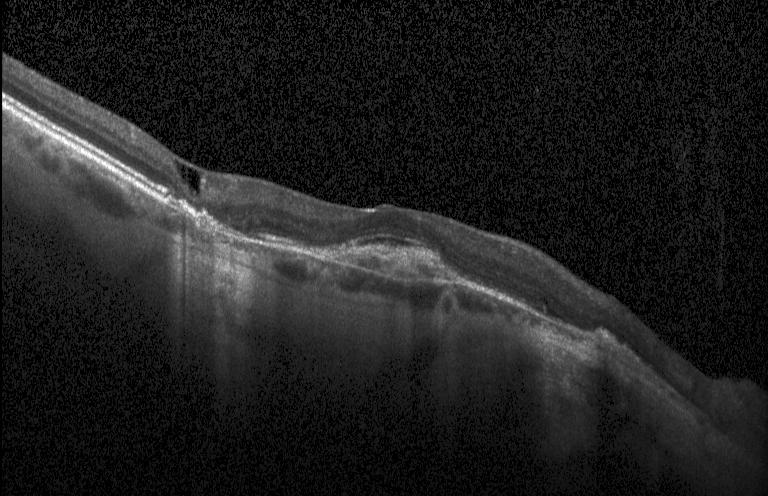 Fovea-centered. OCT B-scan. Spectral-domain optical coherence tomography.
Assessment: a choroidal neovascular membrane.